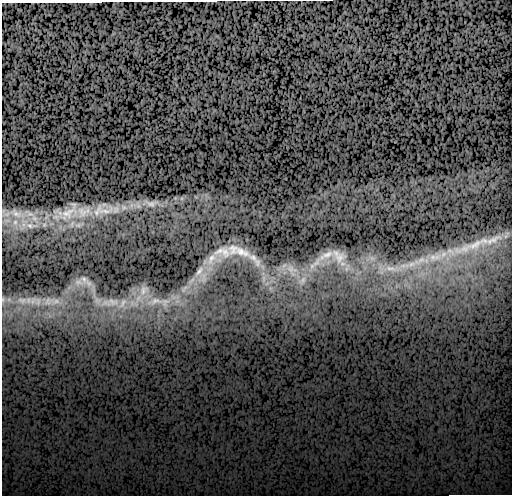 Fovea-centered. Retinal OCT cross-section. Assessment: sub-RPE drusenoid deposits.